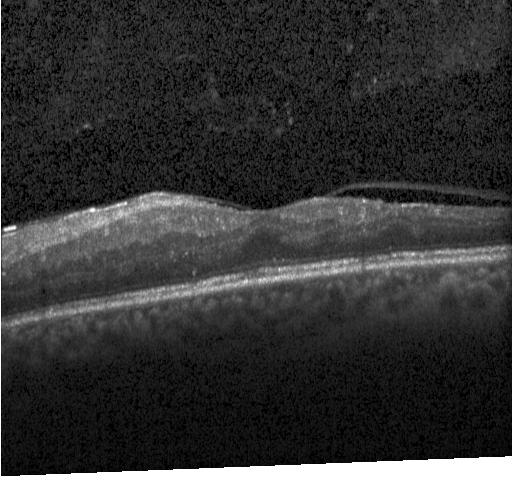 Fovea-centered · OCT B-scan — Dx: diabetic macular edema.